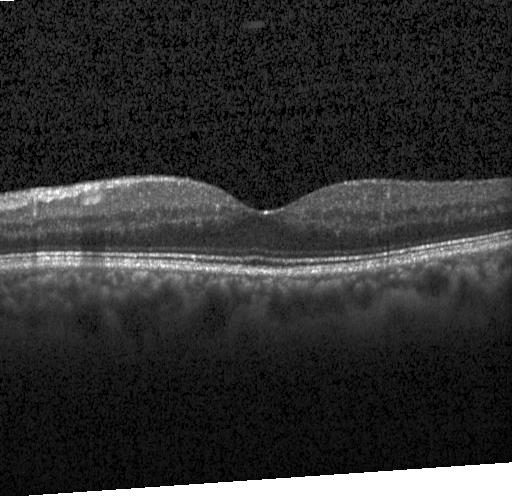
OCT scan showing no choroidal neovascularization, diabetic macular edema, or drusen.